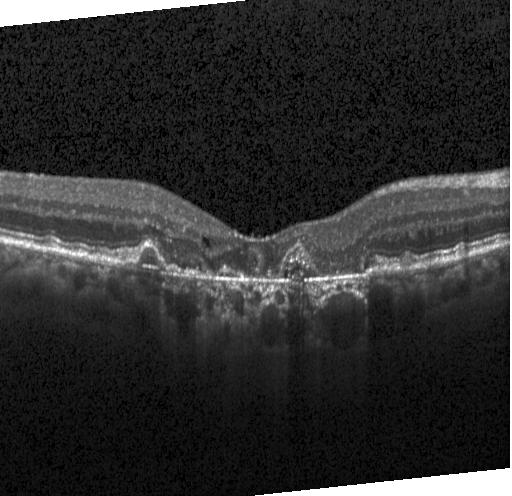 Retinal OCT cross-section showing a choroidal neovascular membrane.